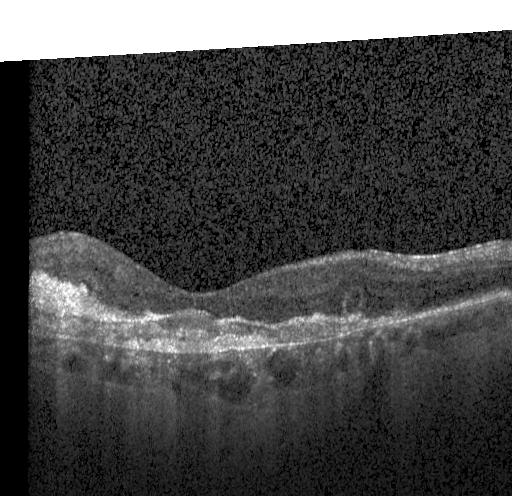
Diagnosis: choroidal neovascularization (CNV).